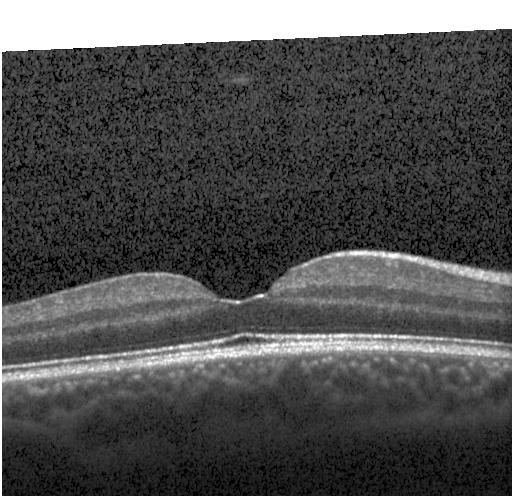
Optical coherence tomography scan. Through the macula — Impression: no CNV, DME, or drusen.